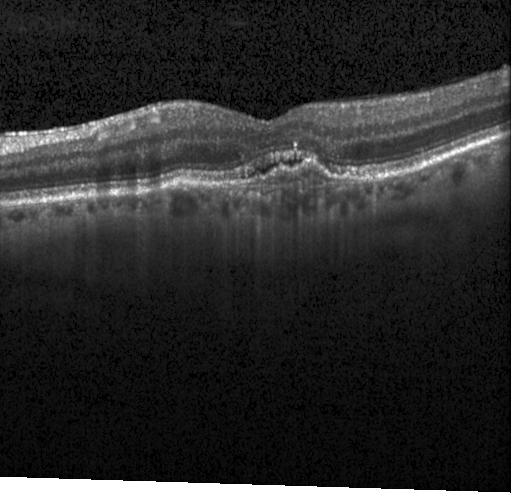 Retinal OCT B-scan · Heidelberg Spectralis OCT system · SD-OCT · macular scan
Impression: a choroidal neovascular membrane.